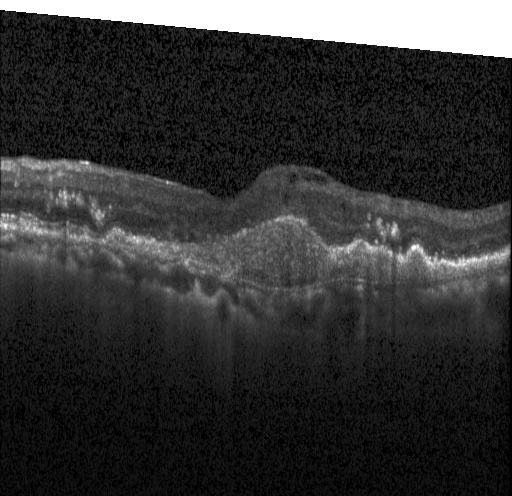

Impression: choroidal neovascularization (CNV).